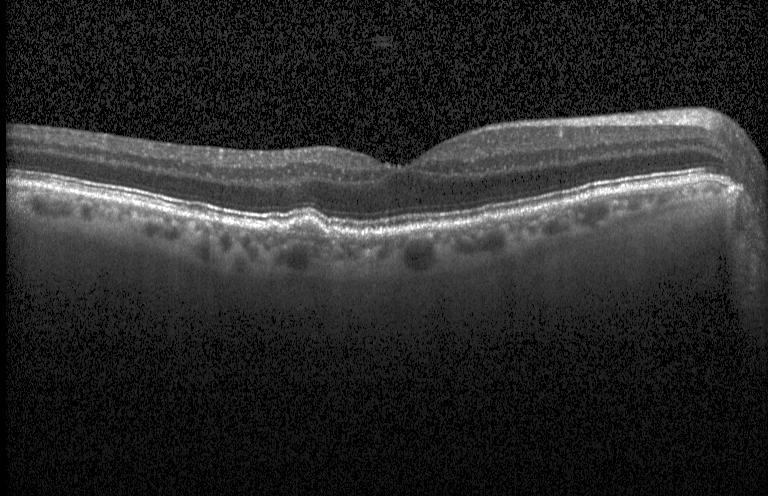 Finding: drusen.